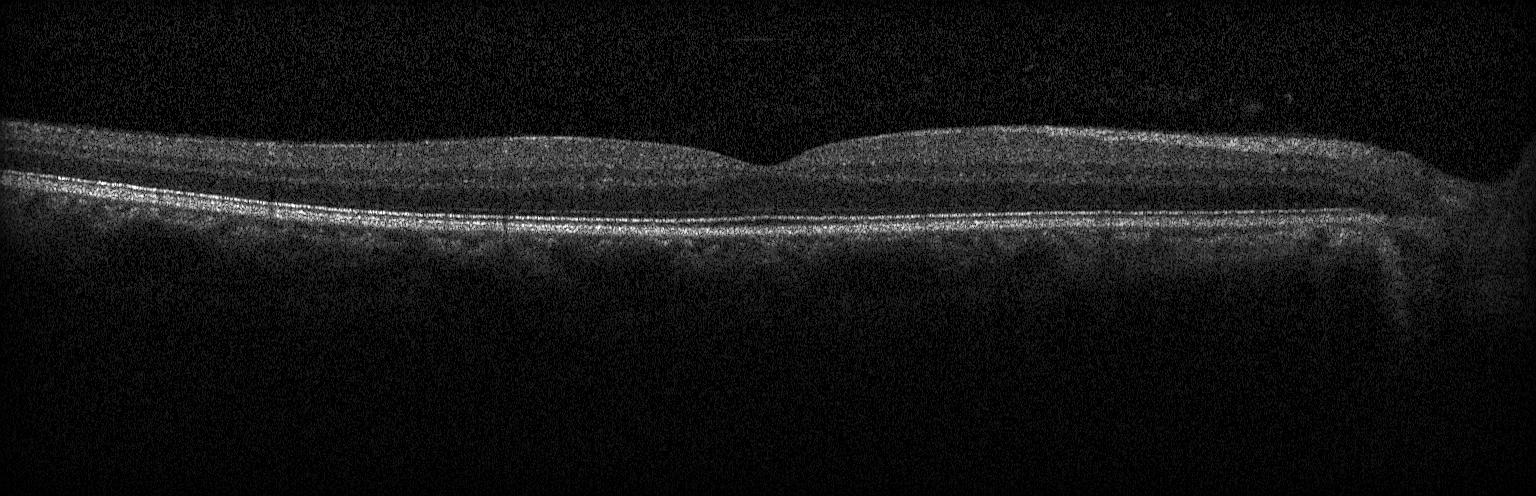
Optical coherence tomography scan, macular scan, acquired on a Heidelberg Spectralis — Dx: neither choroidal neovascularization, diabetic macular edema, nor drusen.